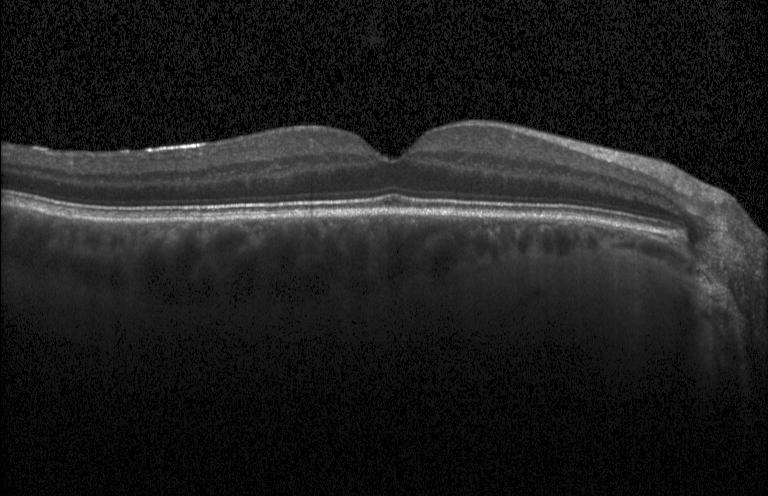
The scan shows no choroidal neovascularization, no diabetic macular edema, and no drusen.